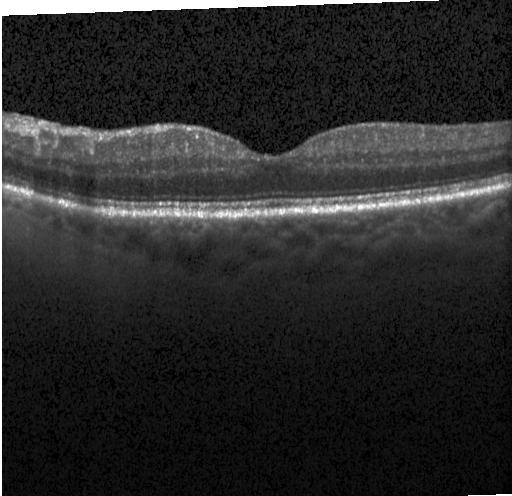
Retinal OCT cross-section. Through the macula.
Impression: no choroidal neovascularization, diabetic macular edema, or drusen.